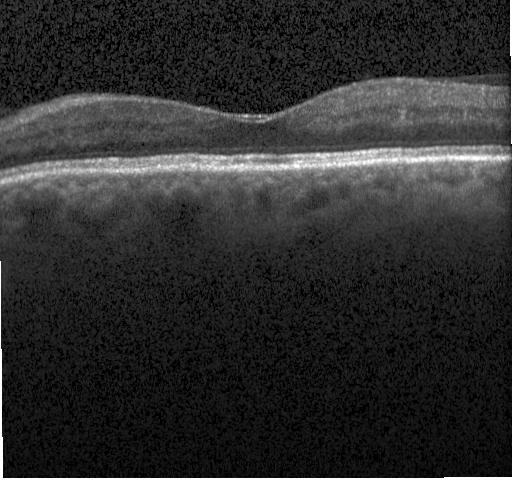 Impression: no choroidal neovascularization, no diabetic macular edema, and no drusen.